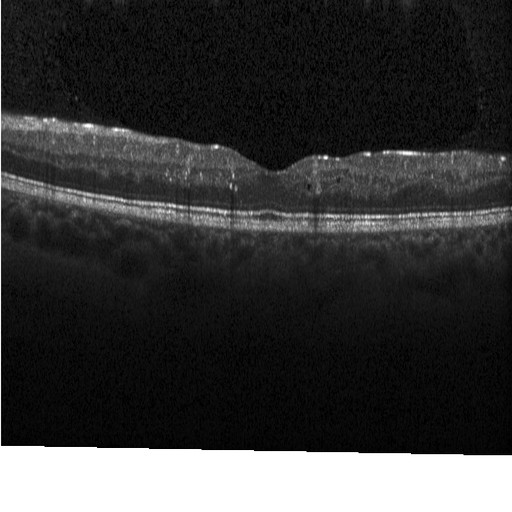

Finding: diabetic macular edema (DME).